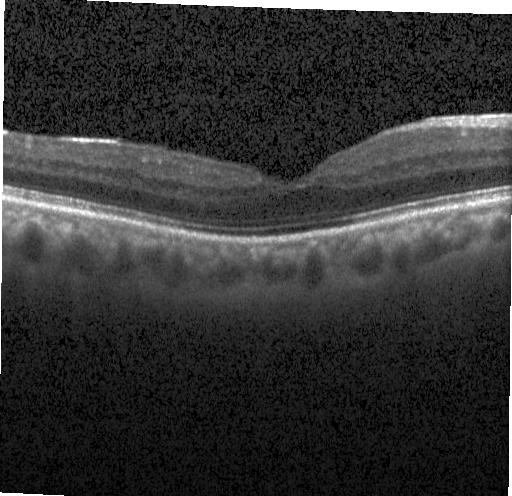

Spectral-domain OCT · OCT line scan · horizontal scan through the fovea
Impression: no choroidal neovascularization, diabetic macular edema, or drusen.